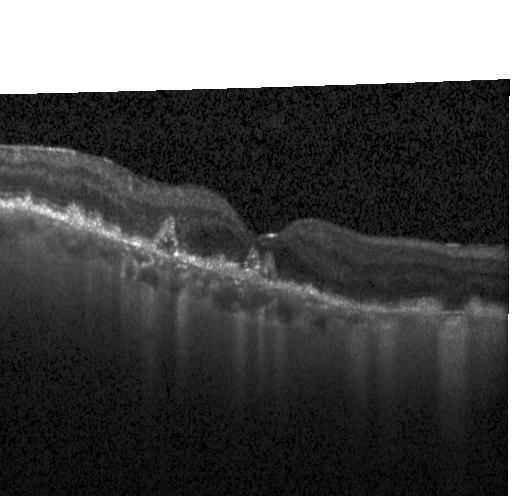
Centered on the fovea · optical coherence tomography B-scan
OCT finding: a choroidal neovascular membrane.